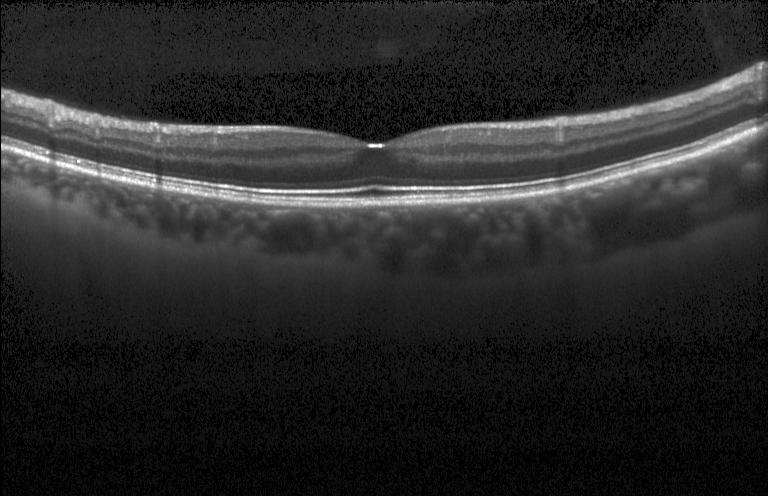

OCT finding: no choroidal neovascularization, no diabetic macular edema, and no drusen.